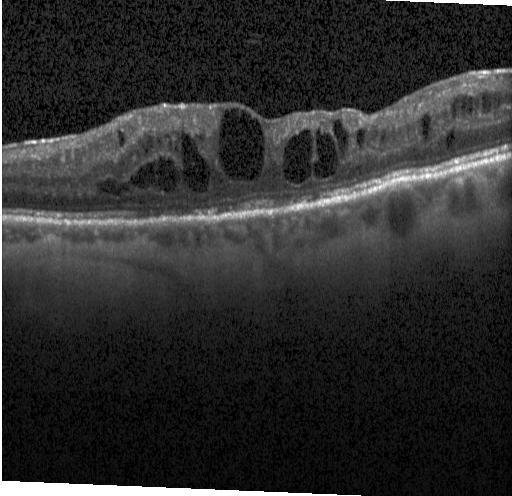

Macular OCT: diabetic macular edema.